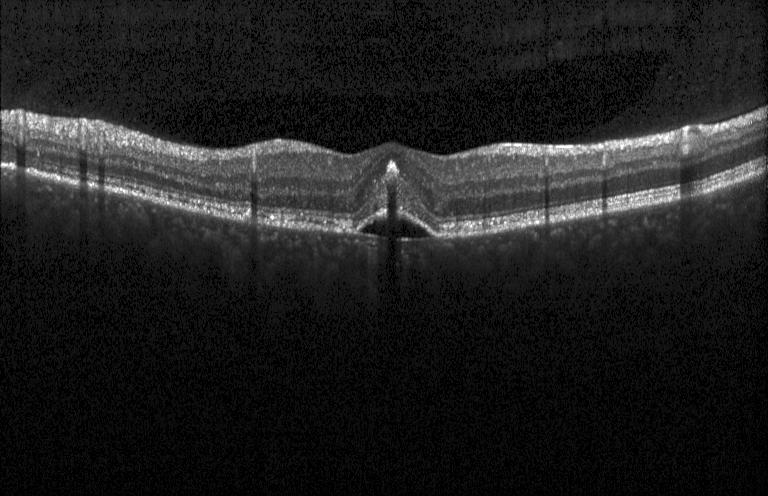 Dx: a choroidal neovascular membrane.